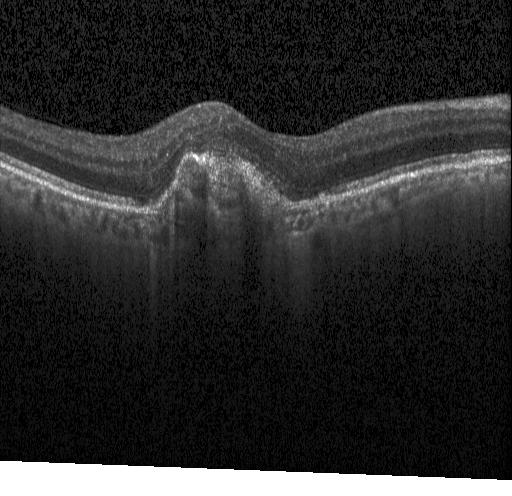 Acquired on a Heidelberg Spectralis. Through the macula. Retinal OCT B-scan — Finding: a choroidal neovascular membrane.